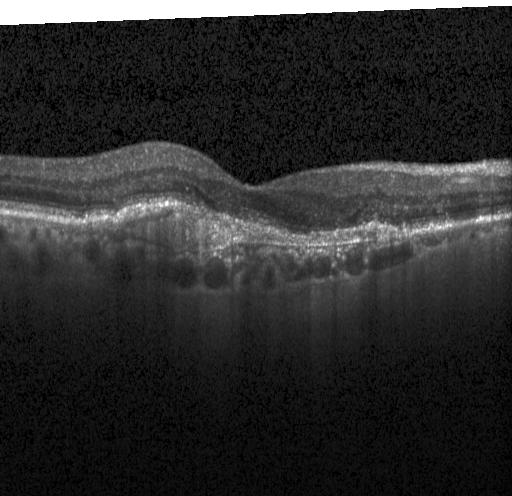

Finding: choroidal neovascularization (CNV).